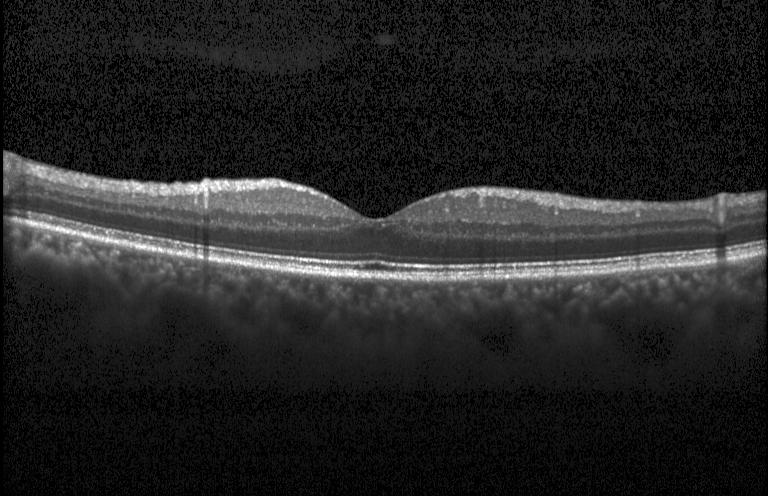 The scan shows no evidence of CNV, DME, or drusen.